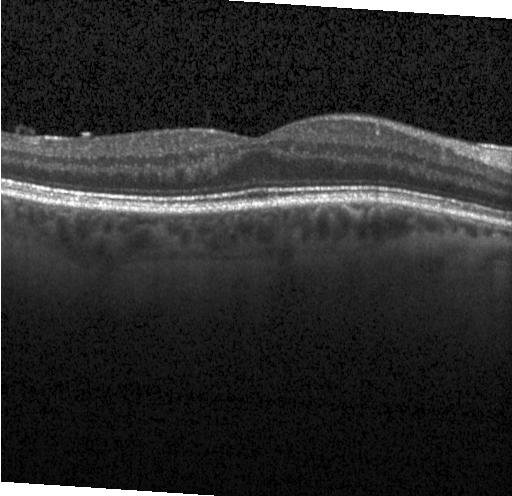 Spectral-domain optical coherence tomography. Heidelberg Spectralis OCT system. Horizontal scan through the fovea. Optical coherence tomography scan. Impression: no evidence of choroidal neovascularization, diabetic macular edema, or drusen.